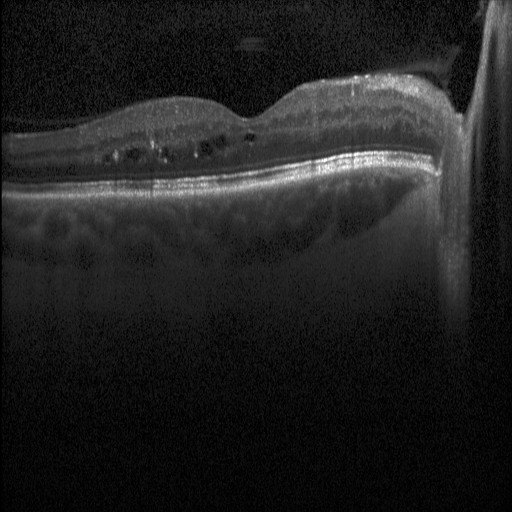

Retinal OCT B-scan, centered on the fovea — Finding: diabetic macular edema.